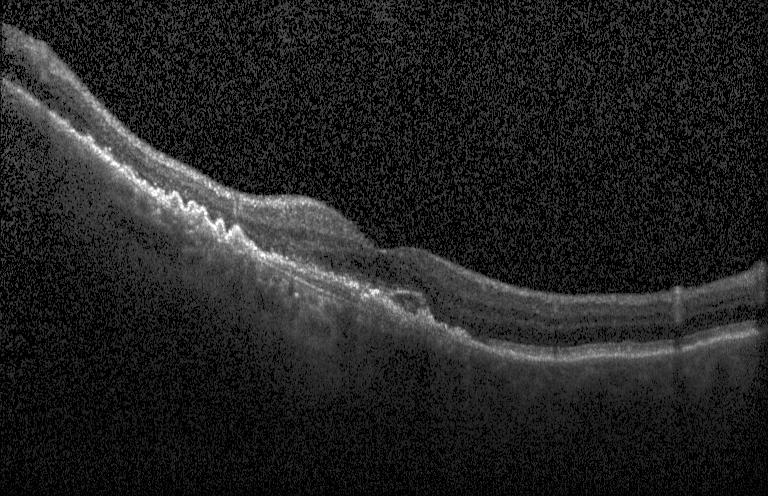
SD-OCT · macular scan · retinal OCT B-scan. OCT finding: a choroidal neovascular membrane.